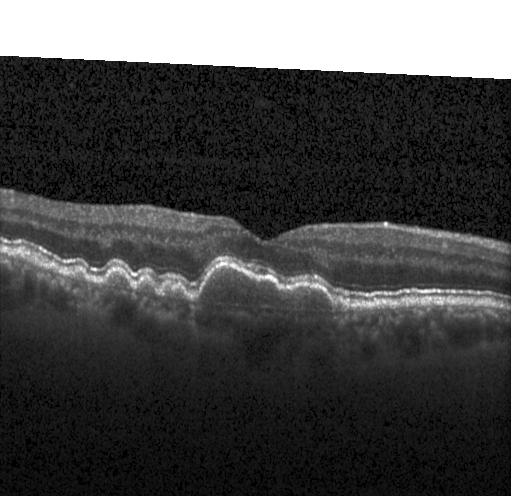

The scan shows drusen.